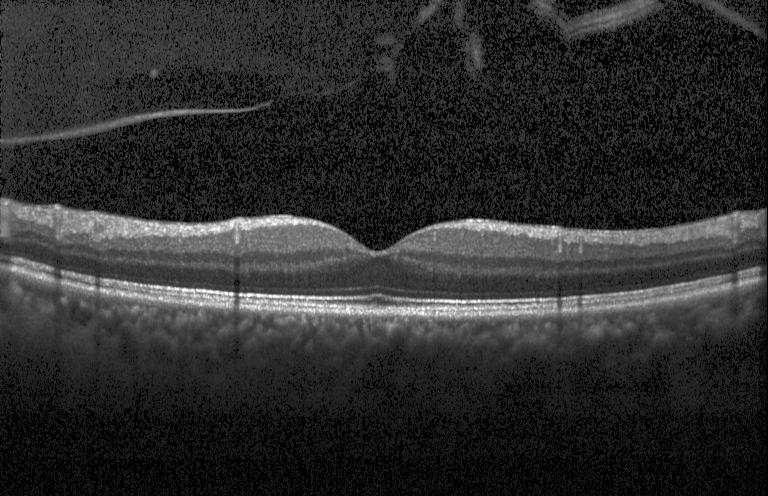
OCT scan showing no evidence of choroidal neovascularization, diabetic macular edema, or drusen.